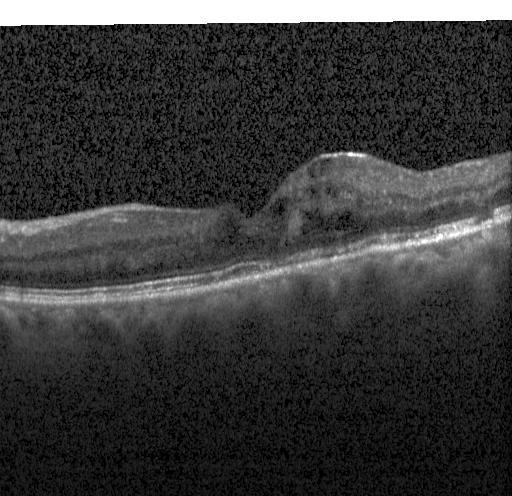

Dx: diabetic macular edema (DME).